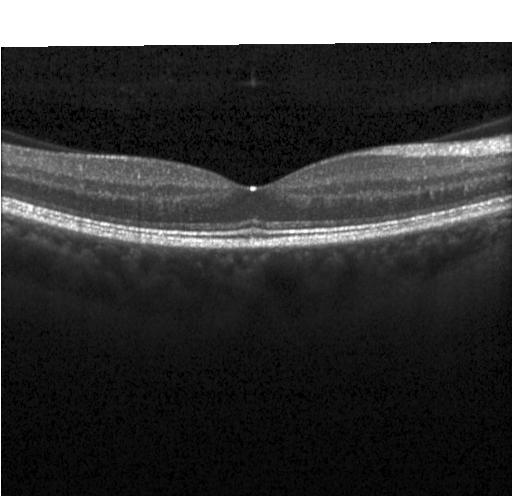 Through the macula; retinal OCT B-scan.
This B-scan demonstrates no choroidal neovascularization, no diabetic macular edema, and no drusen.